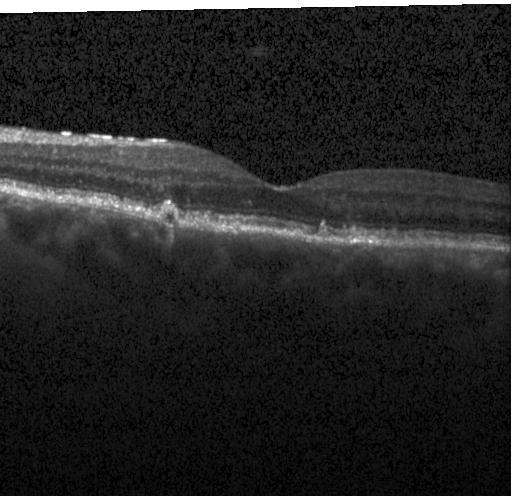
OCT line scan. Fovea-centered. Acquired on a Heidelberg Spectralis — Drusen.